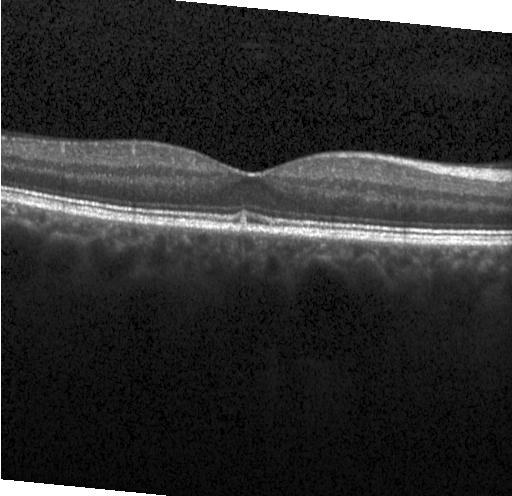 Macular scan, Heidelberg Spectralis OCT system, optical coherence tomography B-scan, spectral-domain optical coherence tomography
This B-scan demonstrates multiple drusen.